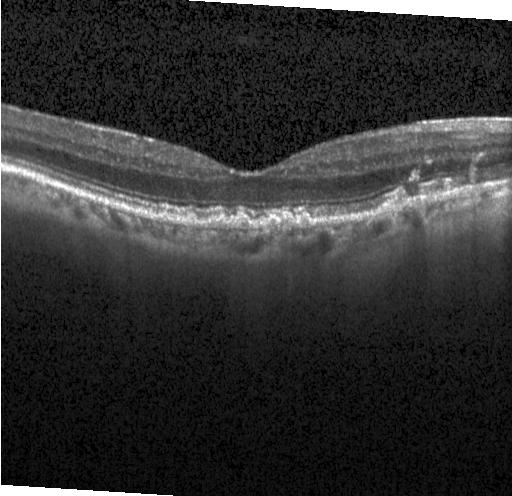 Impression: multiple drusen.